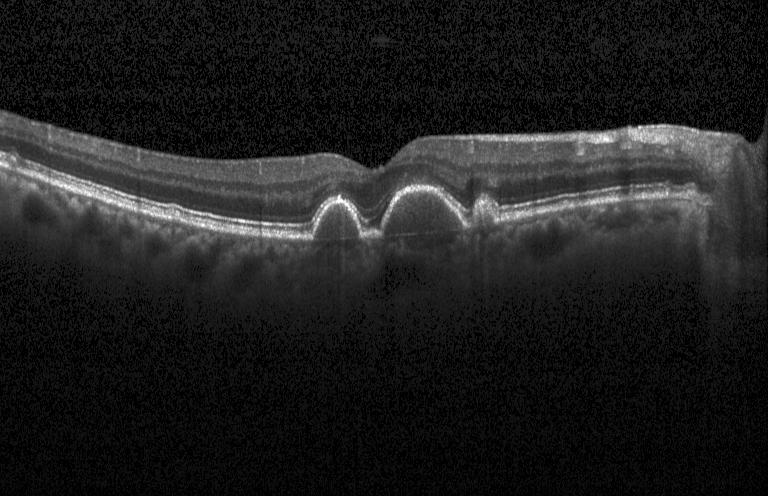
Centered on the fovea, acquired on a Heidelberg Spectralis, optical coherence tomography scan, spectral-domain OCT. The scan shows sub-RPE drusenoid deposits.